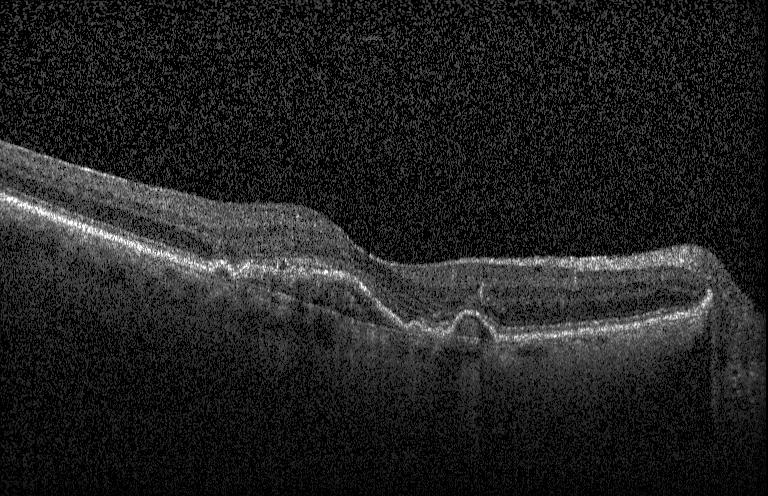
Fovea-centered · optical coherence tomography scan · spectral-domain optical coherence tomography.
OCT finding: a choroidal neovascular membrane.